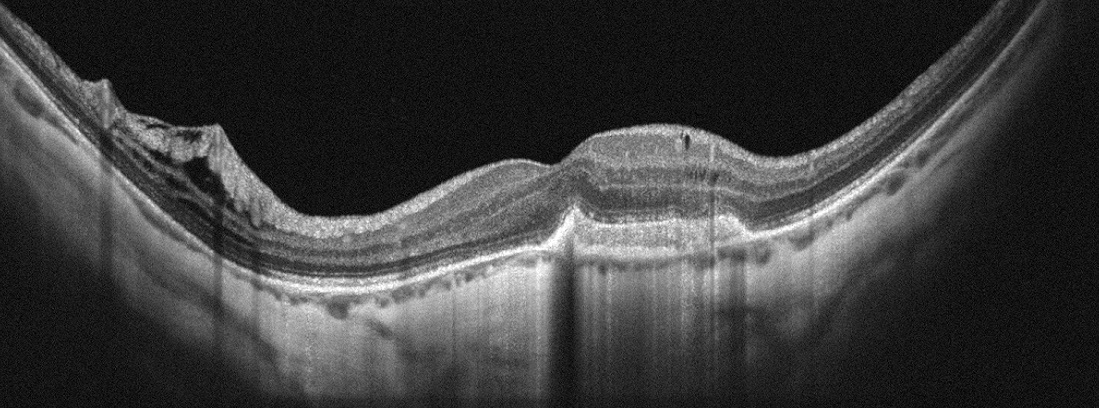
Through the macula; OCT B-scan; Optovue Avanti RTVue XR. Impression: age-related macular degeneration.